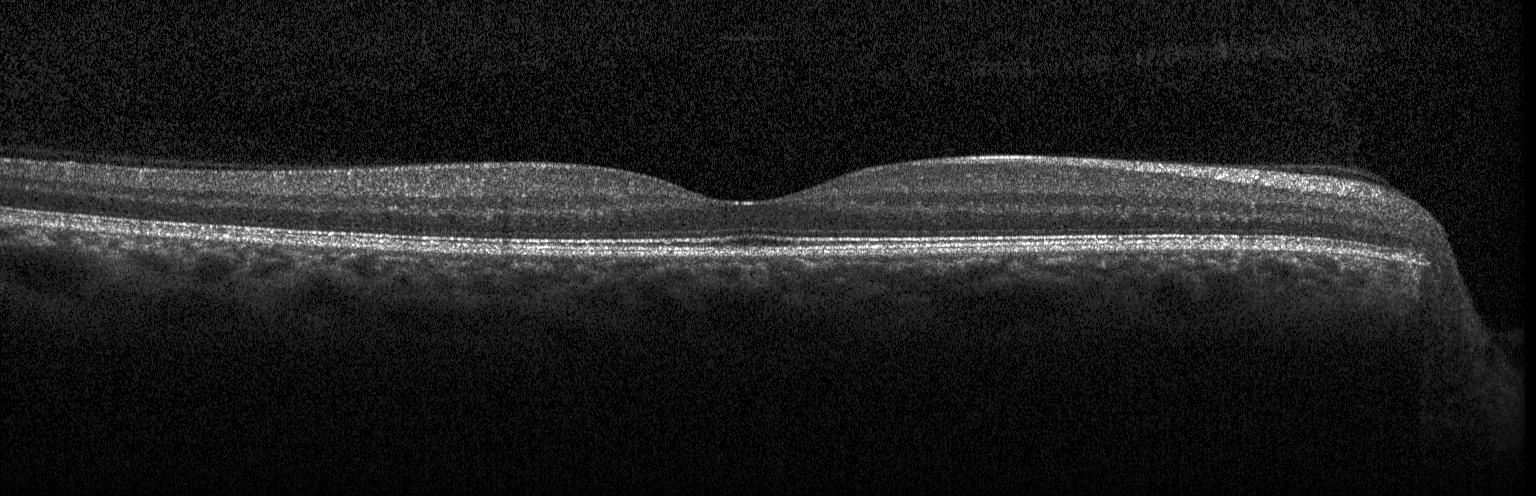
Impression: no choroidal neovascularization, diabetic macular edema, or drusen.